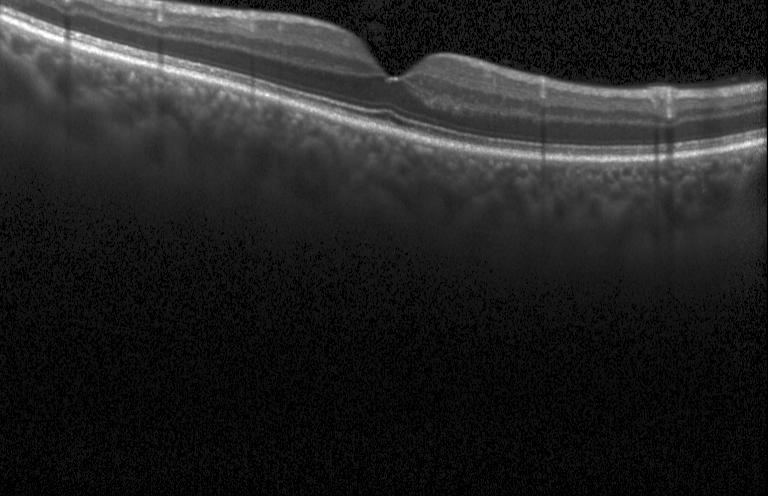

OCT line scan.
Finding: no evidence of choroidal neovascularization, diabetic macular edema, or drusen.